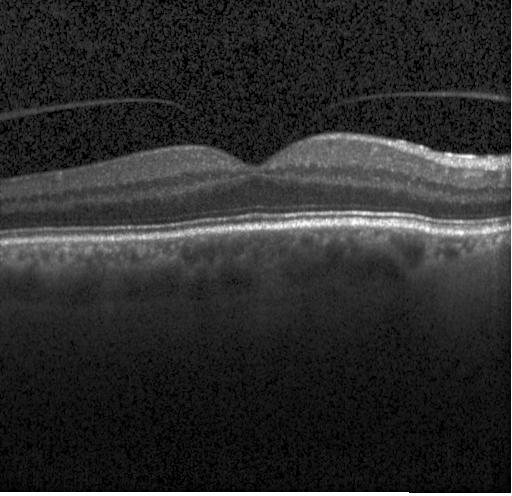

Macular OCT: no choroidal neovascularization, diabetic macular edema, or drusen.